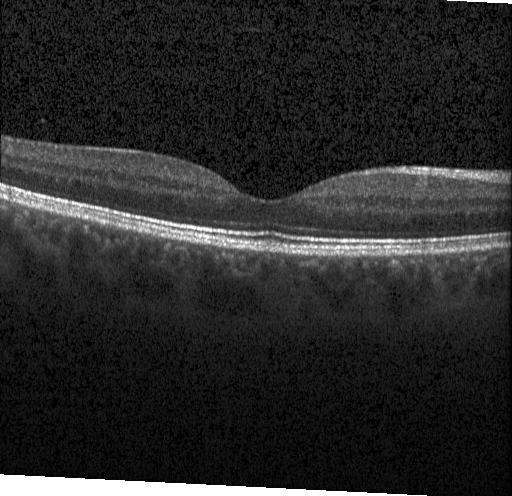

Instrument: Heidelberg Spectralis · macular scan · OCT B-scan
Assessment: no evidence of choroidal neovascularization, diabetic macular edema, or drusen.